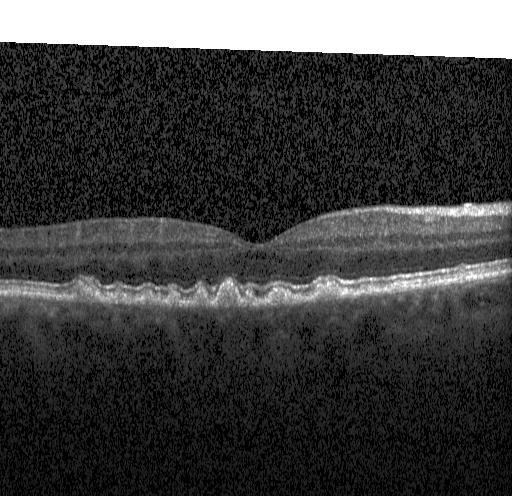
Finding: multiple drusen.